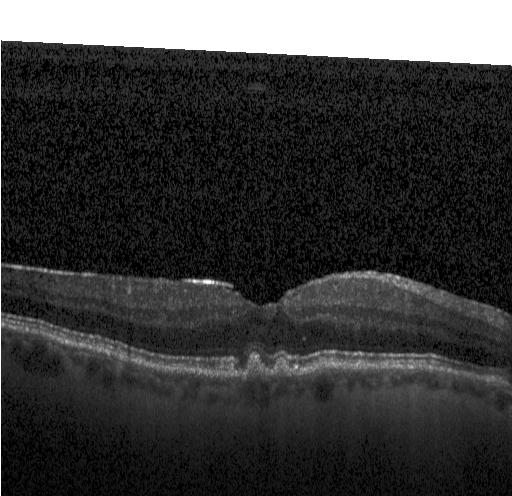
OCT B-scan. Through the macula. SD-OCT. Acquired on a Heidelberg Spectralis
Assessment: sub-RPE drusenoid deposits.